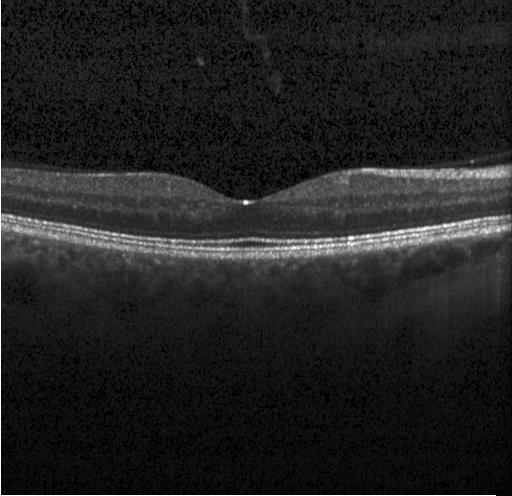

Optical coherence tomography B-scan, spectral-domain optical coherence tomography
Macular OCT: no CNV, no DME, and no drusen.